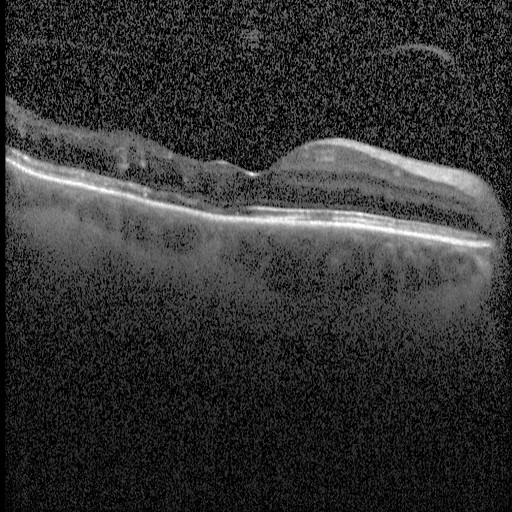
Dx: diabetic macular edema (DME).